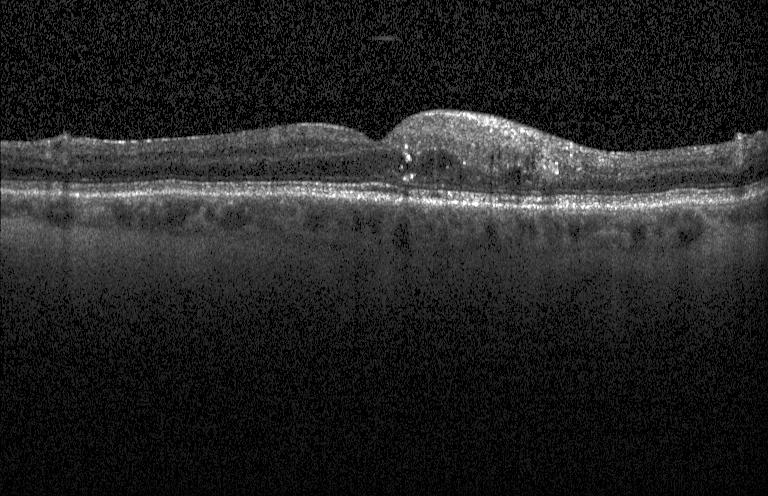 Horizontal scan through the fovea · spectral-domain optical coherence tomography · optical coherence tomography B-scan. This B-scan demonstrates diabetic macular edema (DME).